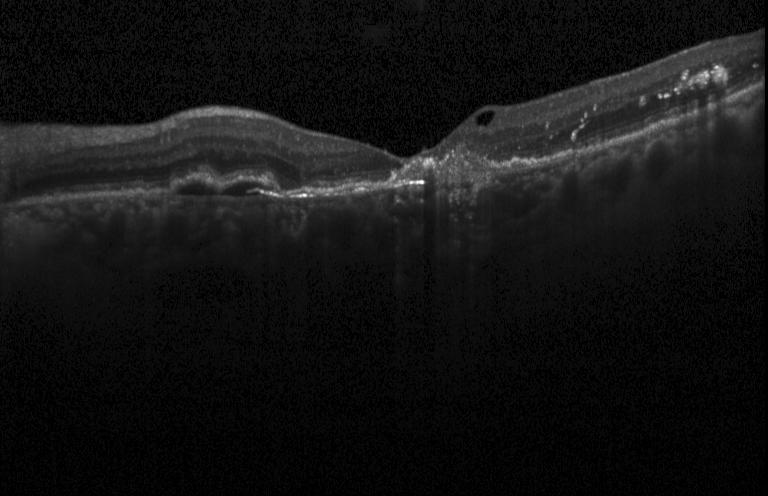

Macular scan, spectral-domain OCT, retinal OCT B-scan.
The scan shows choroidal neovascularization.